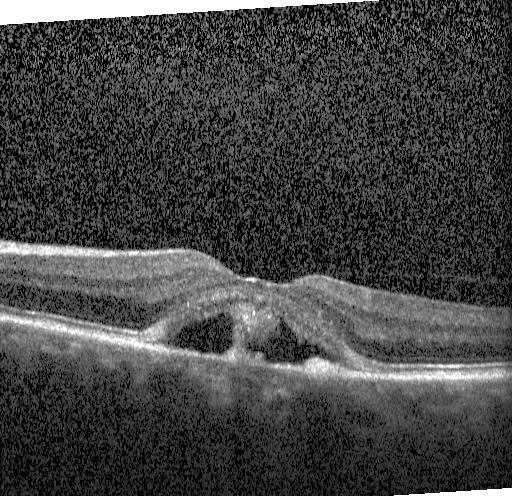
Macular OCT demonstrating choroidal neovascularization (CNV).